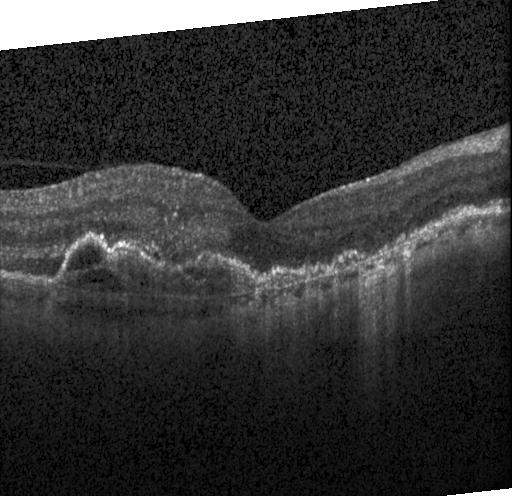

OCT B-scan. Fovea-centered. Heidelberg Spectralis OCT system. Spectral-domain OCT
Choroidal neovascularization (CNV).